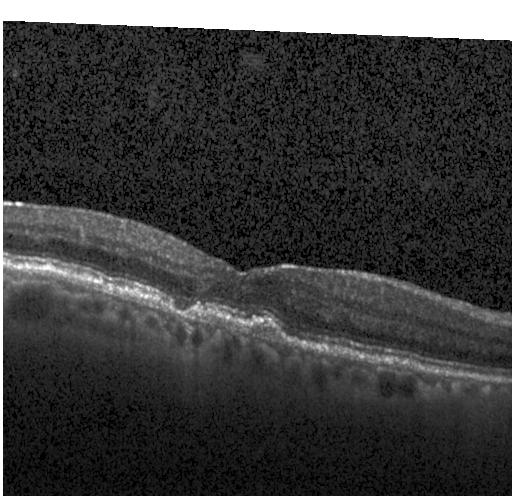
Dx: choroidal neovascularization.